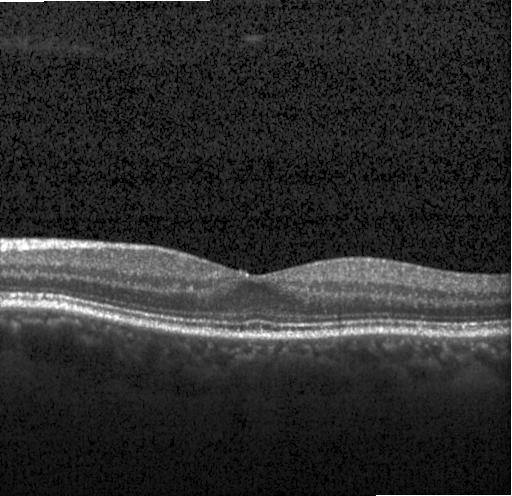 Finding: no evidence of CNV, DME, or drusen.